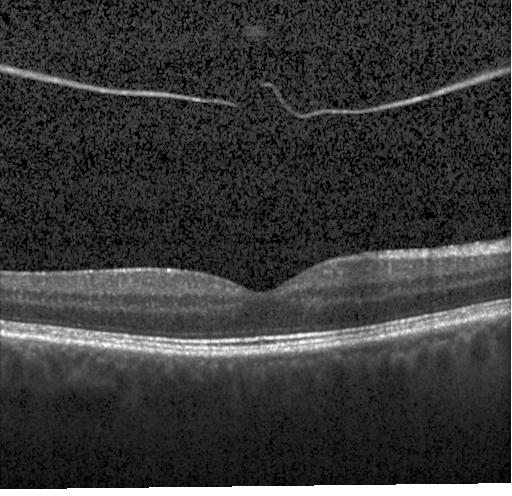 Instrument: Heidelberg Spectralis · fovea-centered · optical coherence tomography B-scan
Dx: neither choroidal neovascularization, diabetic macular edema, nor drusen.